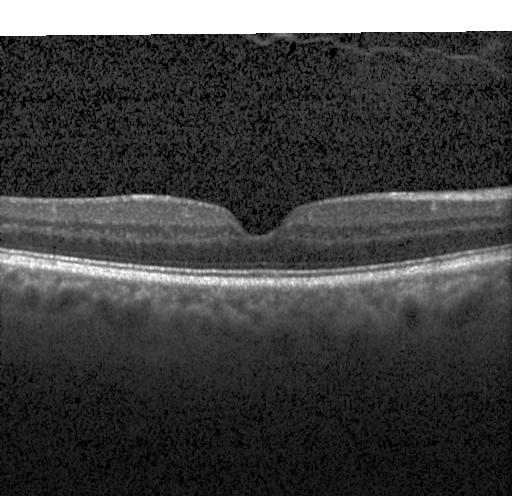 SD-OCT. Heidelberg Spectralis OCT system. Horizontal scan through the fovea. Optical coherence tomography scan. Assessment: no choroidal neovascularization, diabetic macular edema, or drusen.